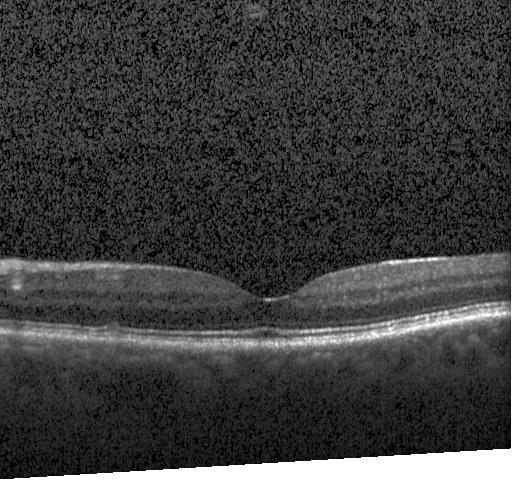
OCT line scan — This B-scan demonstrates no choroidal neovascularization, no diabetic macular edema, and no drusen.